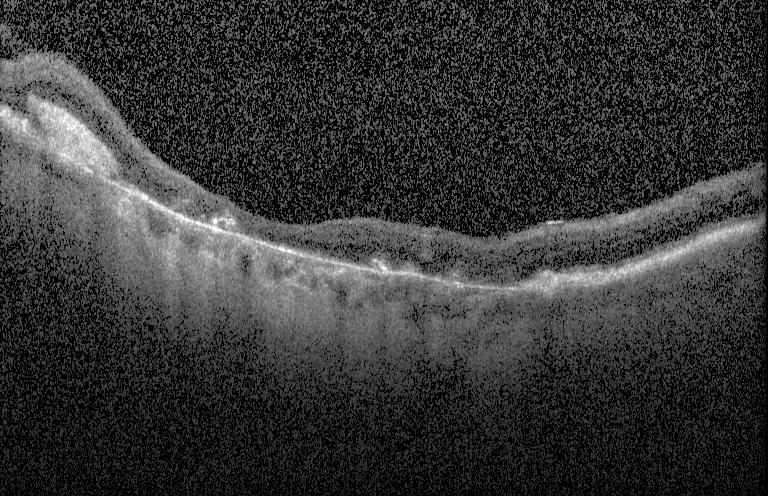 Finding: a choroidal neovascular membrane.